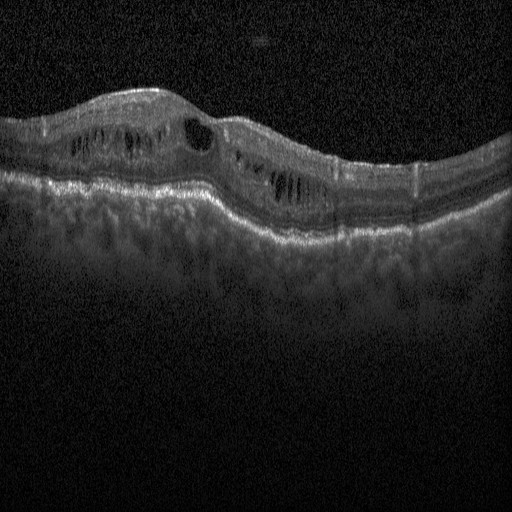
Assessment: diabetic macular edema (DME).